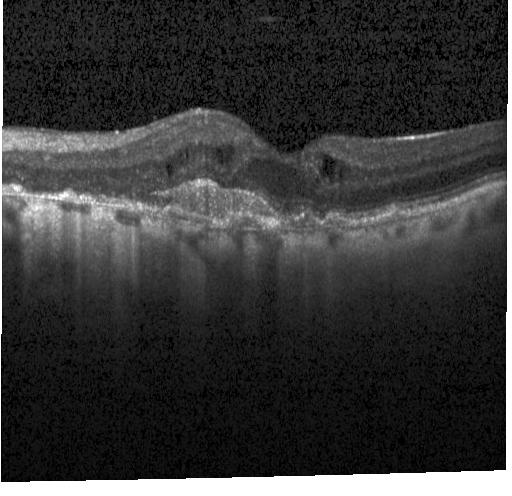 Fovea-centered; optical coherence tomography B-scan; Heidelberg Spectralis; spectral-domain OCT.
Diagnosis: a choroidal neovascular membrane.